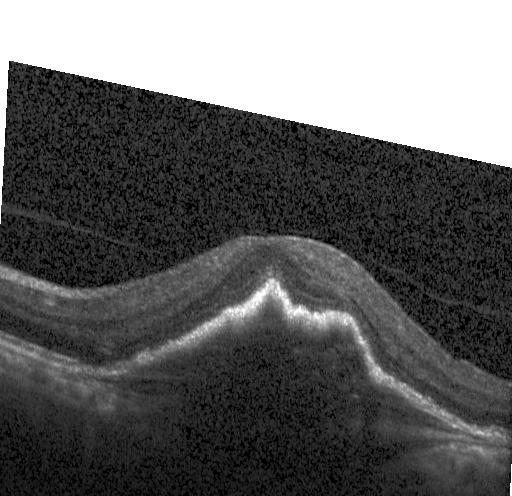

Dx: choroidal neovascularization (CNV).